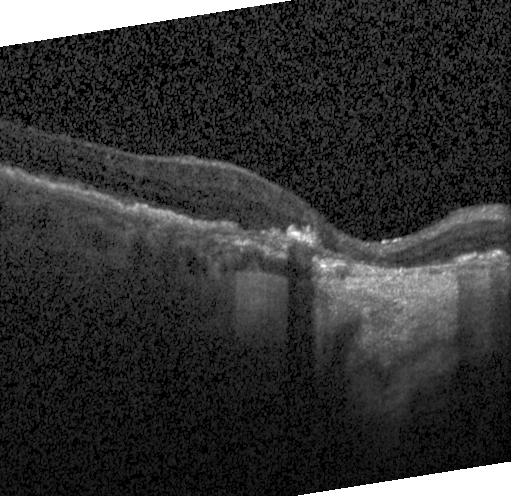 Macular scan; optical coherence tomography B-scan; Heidelberg Spectralis — CNV.